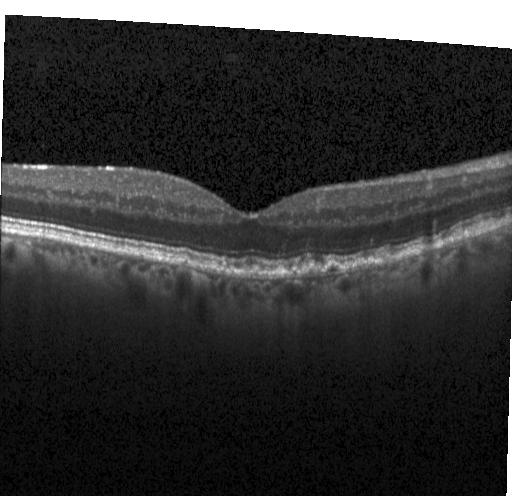 Diagnosis: drusen.